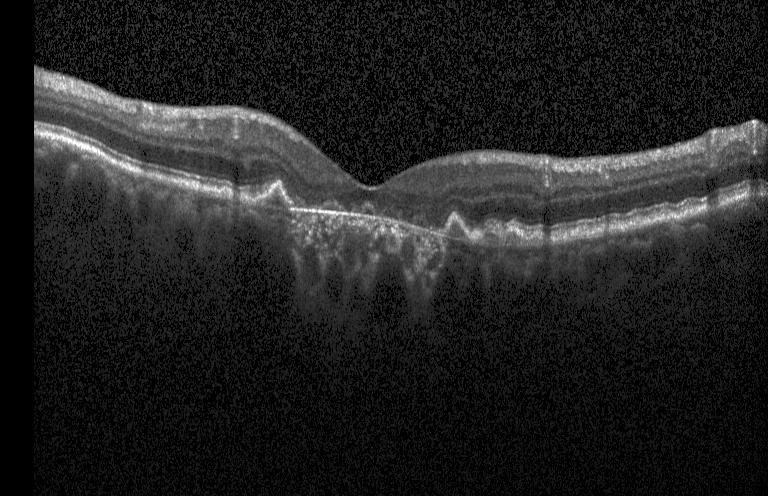

OCT line scan — A choroidal neovascular membrane.